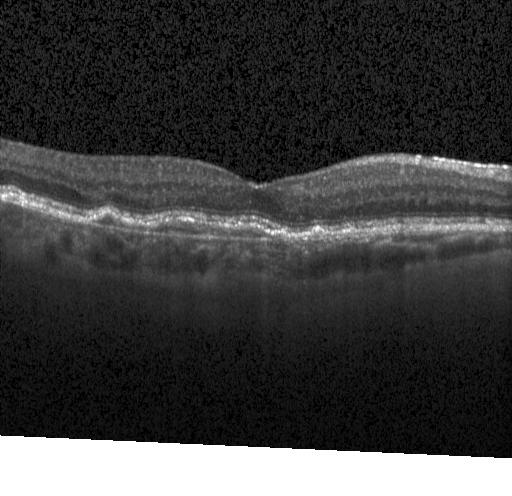
Optical coherence tomography scan.
Diagnosis: a choroidal neovascular membrane.